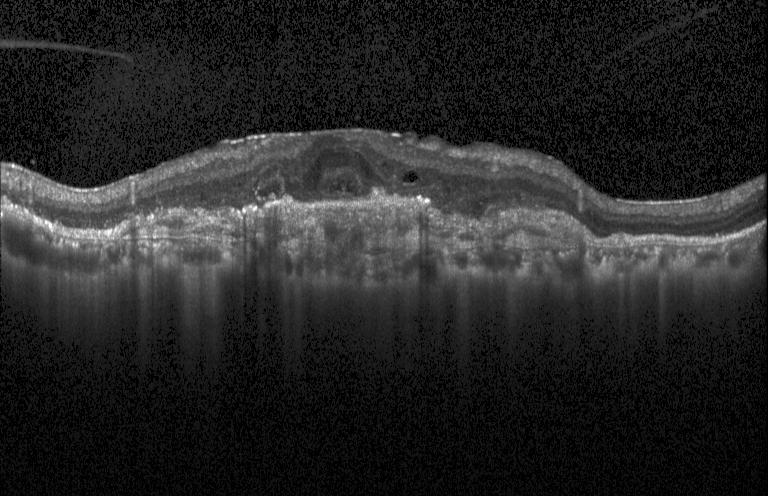

Spectral-domain OCT. Through the macula. Optical coherence tomography B-scan — Diagnosis: choroidal neovascularization (CNV).